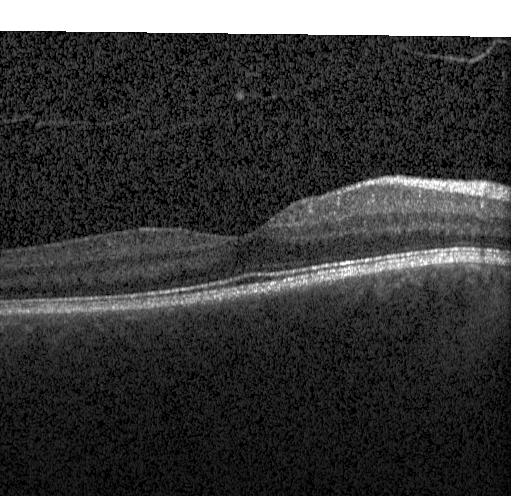

Centered on the fovea, spectral-domain OCT, OCT B-scan
Impression: no choroidal neovascularization, diabetic macular edema, or drusen.